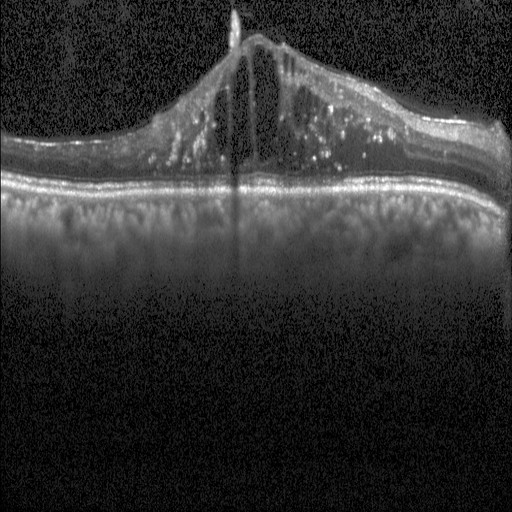 Retinal OCT cross-section — Assessment: diabetic macular edema (DME).